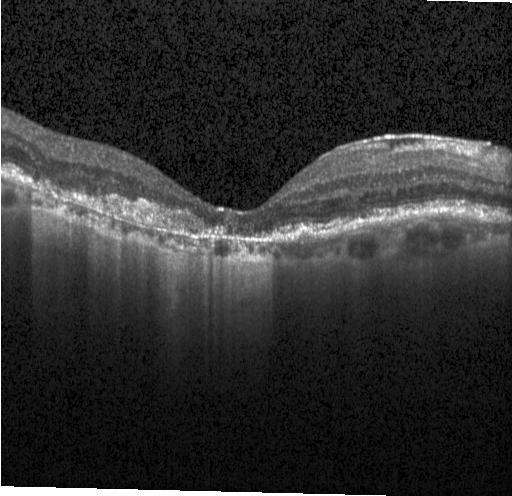

OCT line scan; centered on the fovea
OCT finding: choroidal neovascularization (CNV).